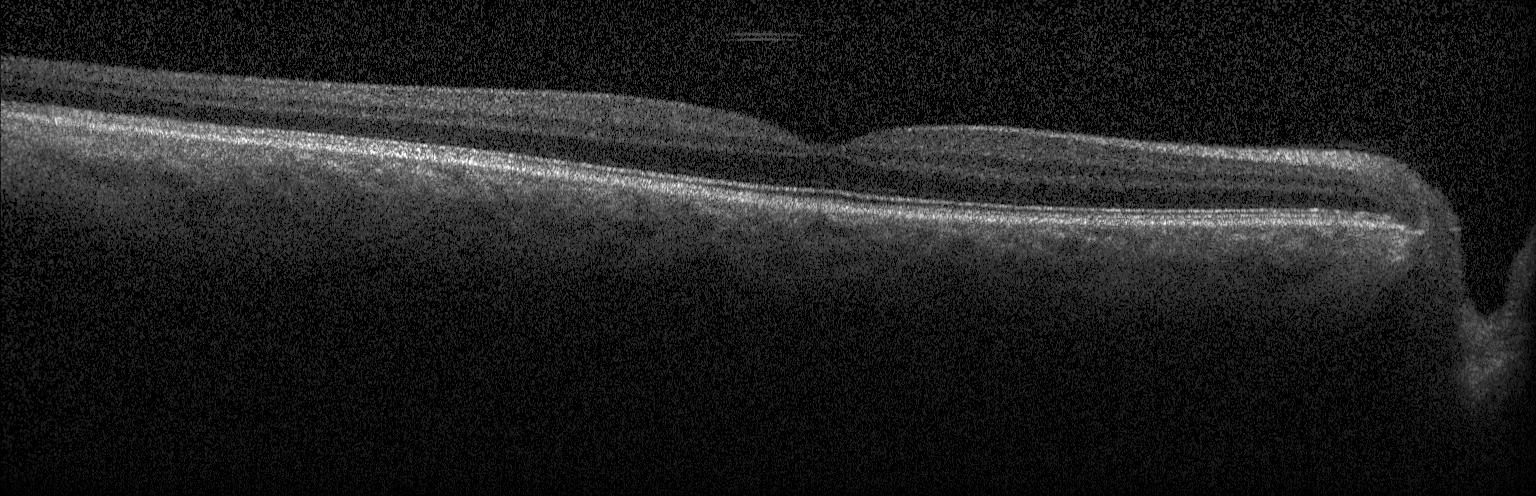
OCT line scan
Impression: no choroidal neovascularization, diabetic macular edema, or drusen.